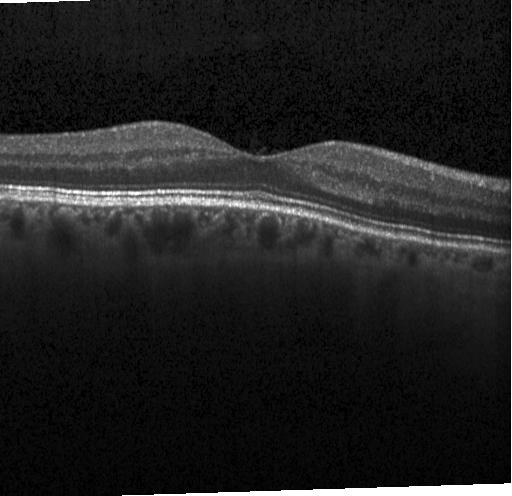
Heidelberg Spectralis OCT system, fovea-centered, retinal OCT B-scan
OCT finding: no CNV, no DME, and no drusen.